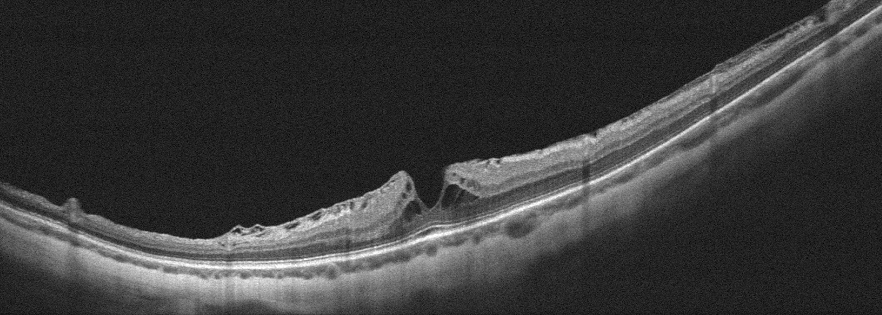
Fovea-centered; retinal OCT cross-section; OS — VID.